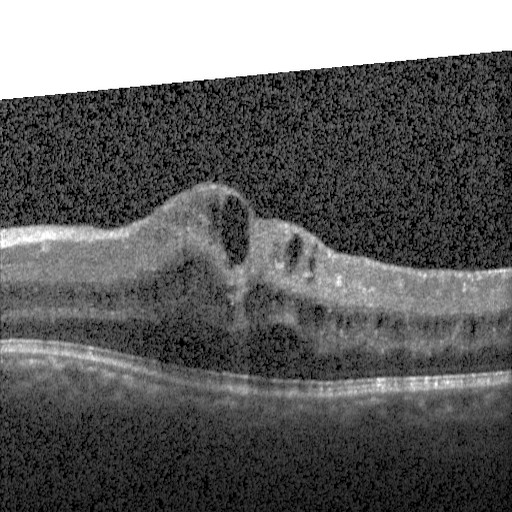

Retinal OCT B-scan; centered on the fovea; SD-OCT — The scan shows diabetic macular edema (DME).